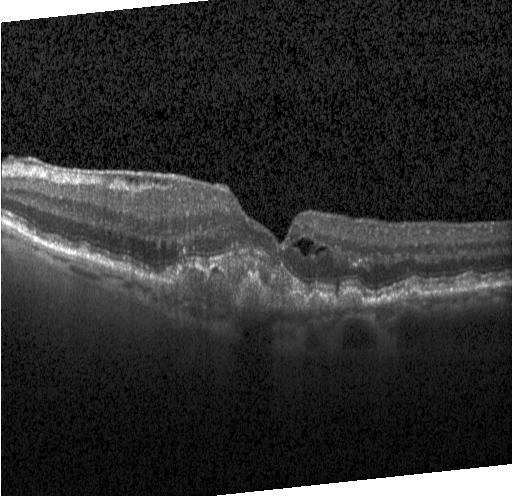 Finding: a choroidal neovascular membrane.